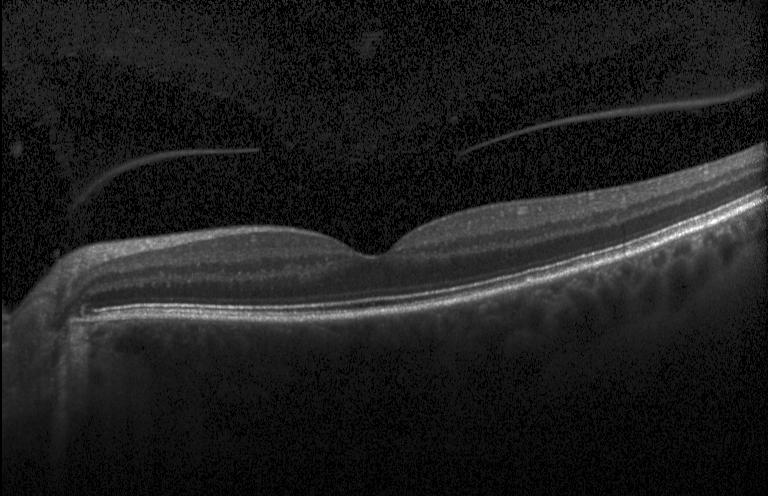 Spectral-domain OCT · retinal OCT cross-section.
Finding: neither choroidal neovascularization, diabetic macular edema, nor drusen.